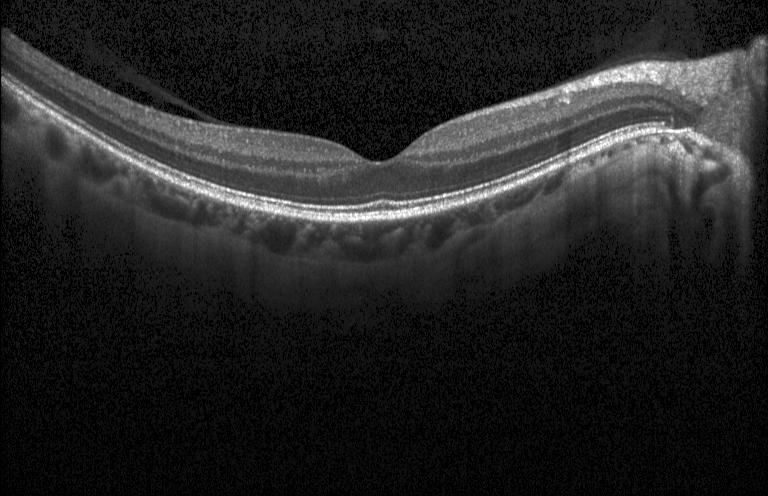 OCT line scan. Spectral-domain optical coherence tomography — No choroidal neovascularization, no diabetic macular edema, and no drusen.